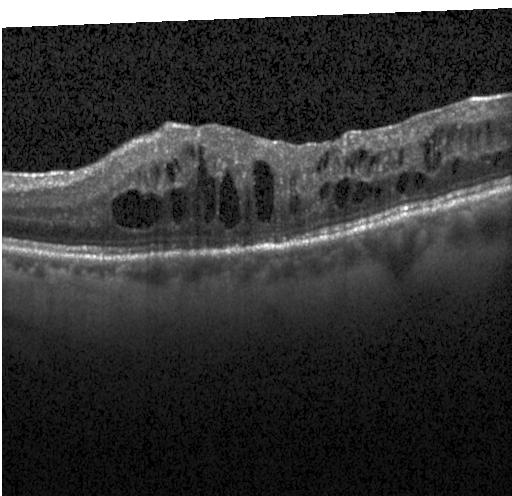 OCT B-scan; through the macula.
Diagnosis: diabetic macular edema (DME).